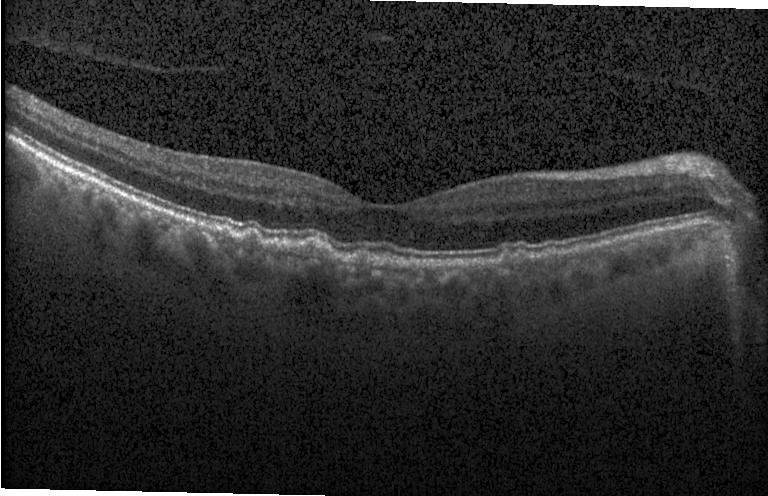
OCT B-scan showing multiple drusen.